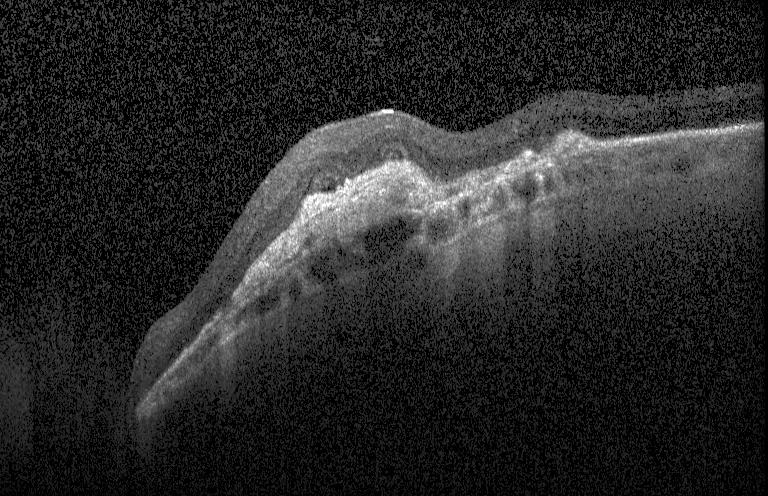
OCT B-scan. Spectral-domain OCT.
Assessment: choroidal neovascularization (CNV).